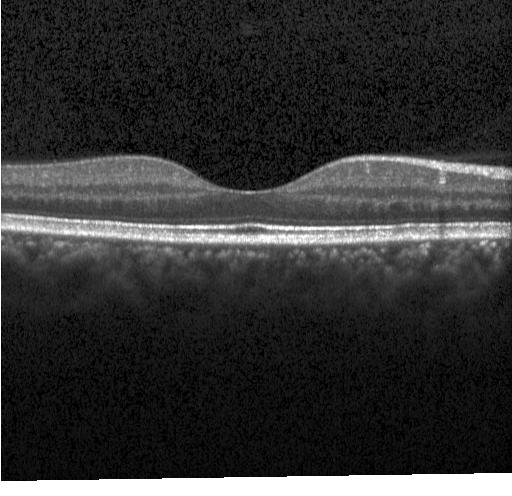
Retinal OCT B-scan
The scan shows no evidence of CNV, DME, or drusen.